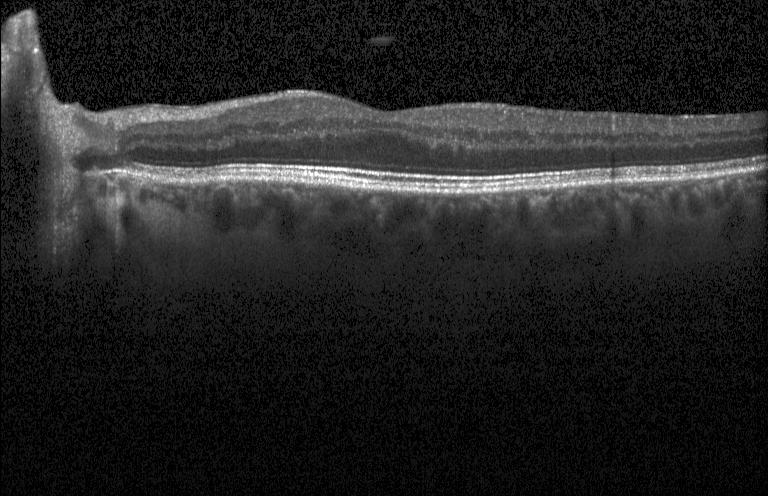
Retinal OCT B-scan. Heidelberg Spectralis. Through the macula. Spectral-domain optical coherence tomography. Impression: no CNV, no DME, and no drusen.